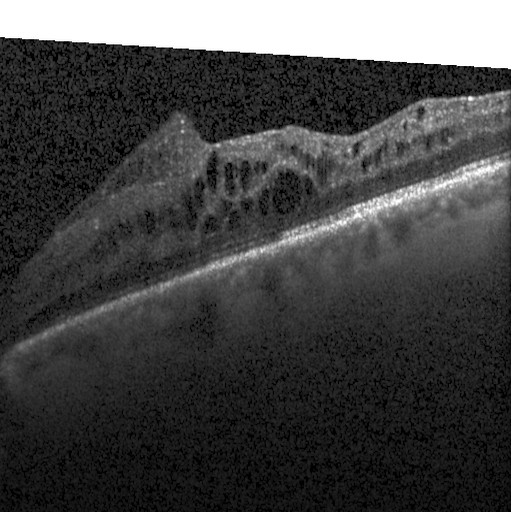
Dx: diabetic macular edema (DME).